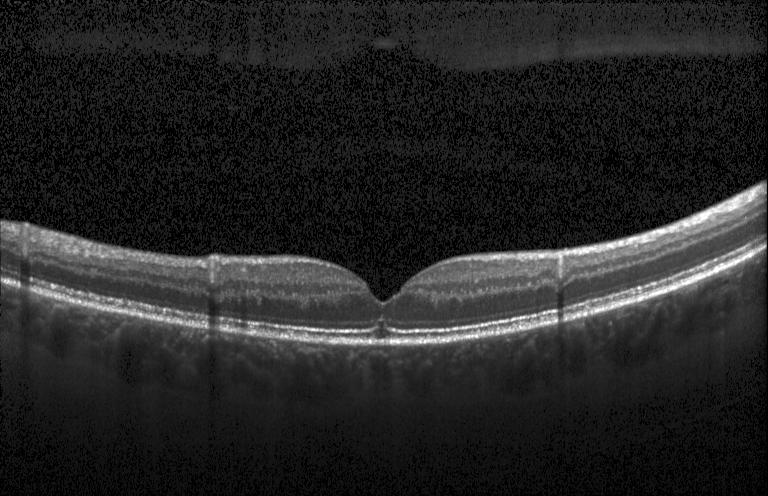

Spectral-domain OCT B-scan: no CNV, DME, or drusen.